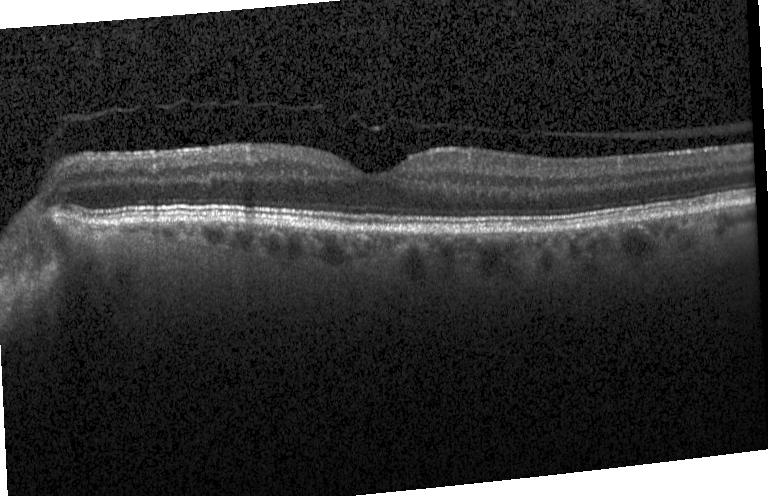 OCT scan showing neither choroidal neovascularization, diabetic macular edema, nor drusen.